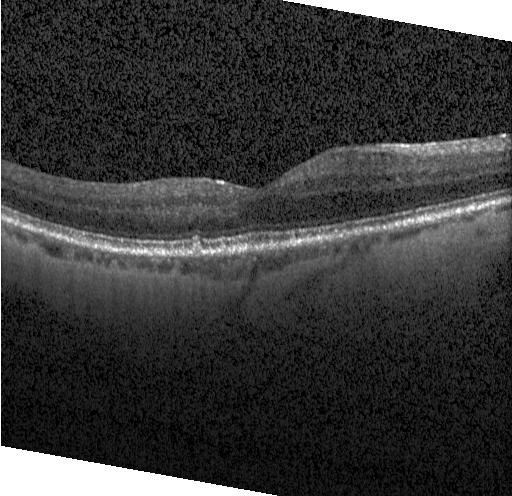
Spectral-domain OCT B-scan: multiple drusen.